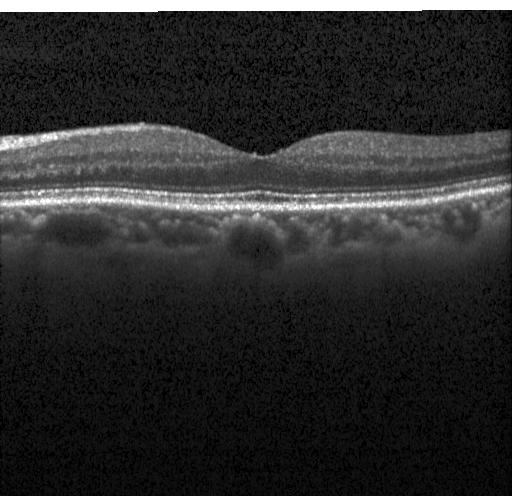
Fovea-centered, retinal OCT B-scan, Heidelberg Spectralis OCT system, spectral-domain OCT. The scan shows no choroidal neovascularization, no diabetic macular edema, and no drusen.